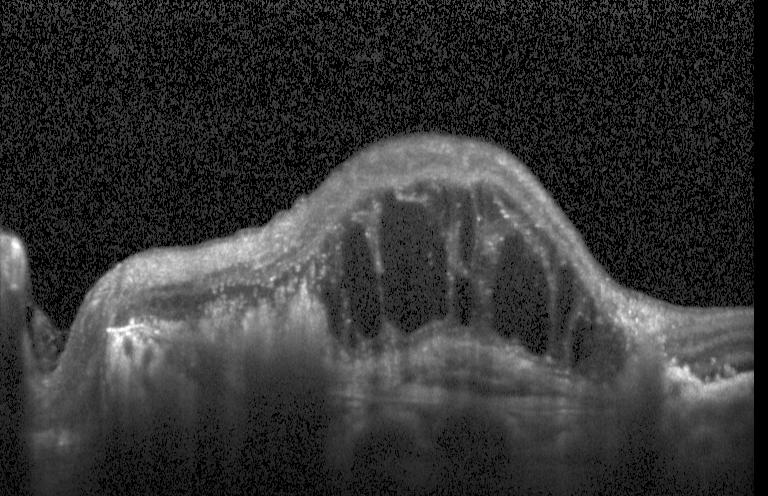
Impression: a choroidal neovascular membrane.